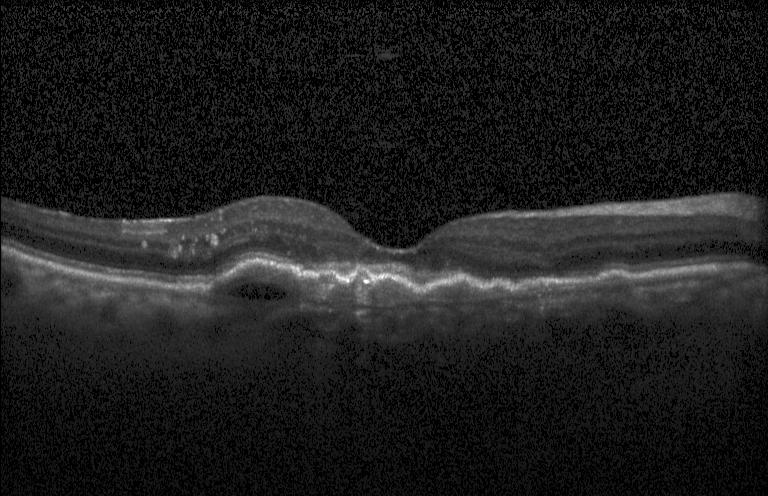

Retinal OCT cross-section · spectral-domain optical coherence tomography.
Finding: a choroidal neovascular membrane.